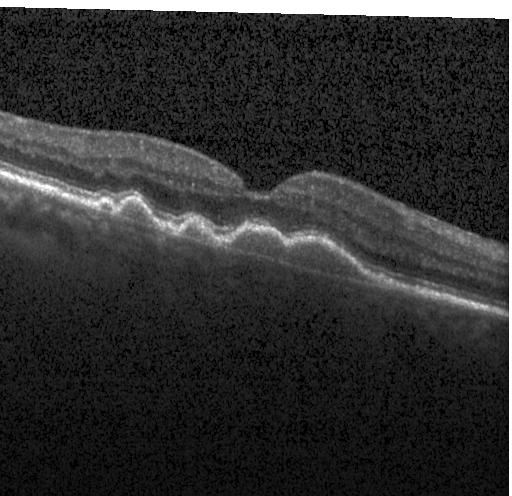 Optical coherence tomography B-scan.
Impression: CNV.